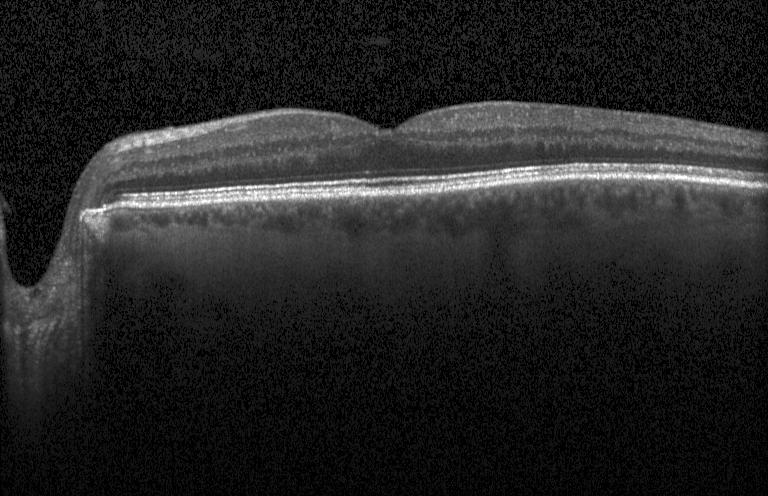 Spectral-domain OCT; retinal OCT cross-section.
Finding: no choroidal neovascularization, no diabetic macular edema, and no drusen.